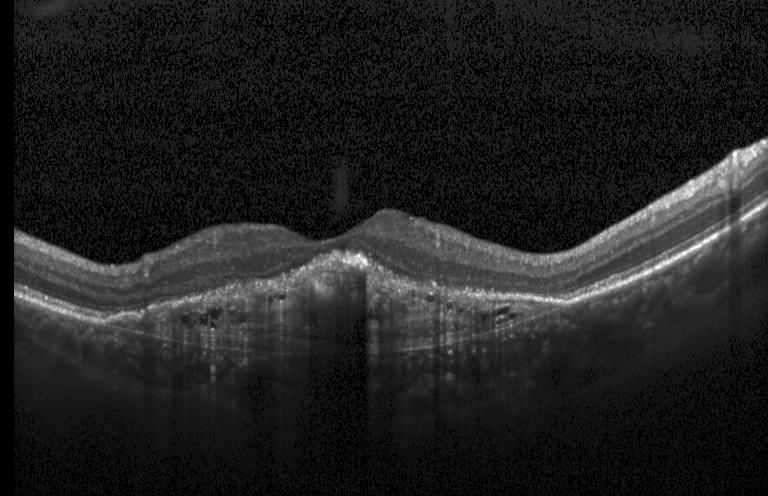

Spectral-domain OCT B-scan: a choroidal neovascular membrane.